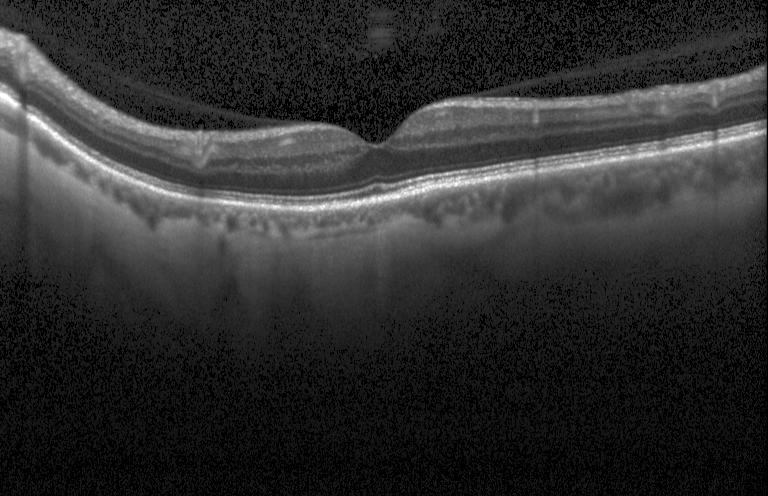 Optical coherence tomography scan — Finding: no CNV, DME, or drusen.